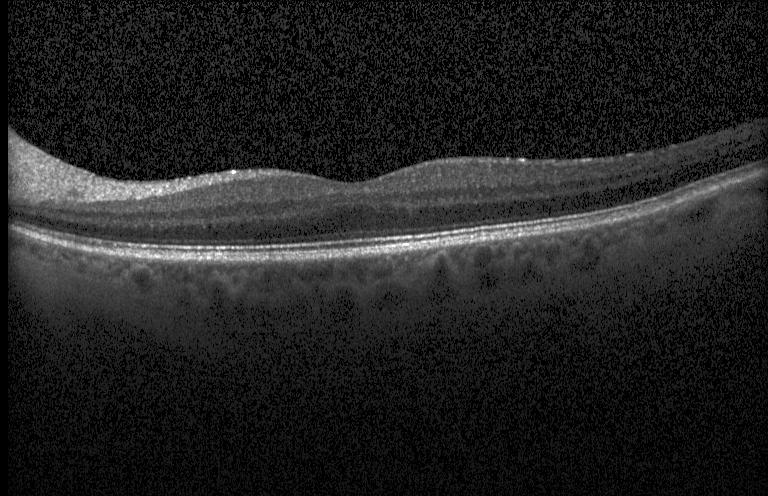
Optical coherence tomography scan
Diagnosis: no choroidal neovascularization, diabetic macular edema, or drusen.